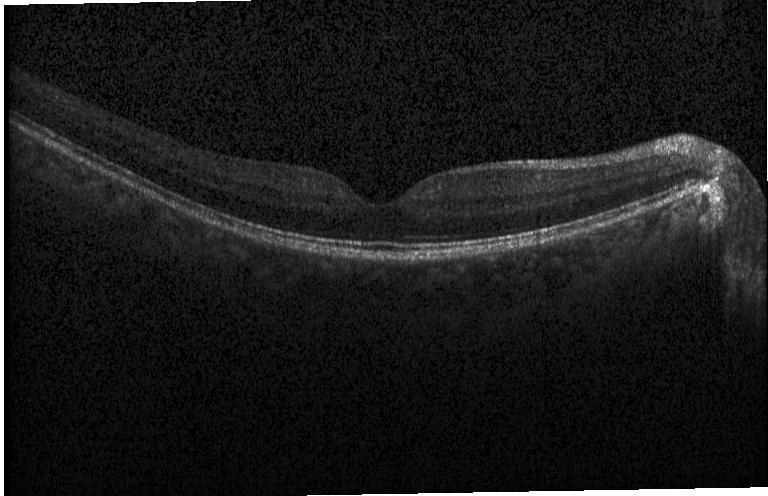

Finding: no choroidal neovascularization, diabetic macular edema, or drusen.